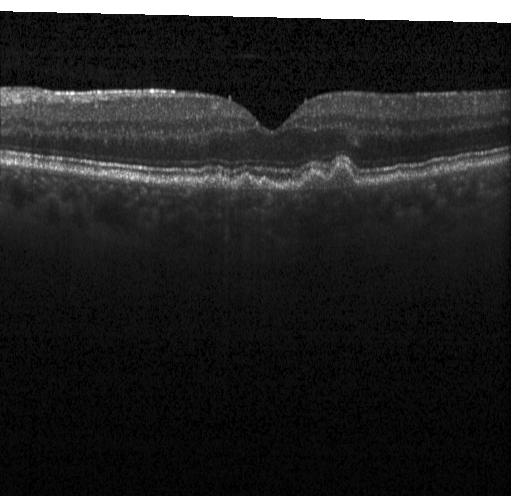
Retinal OCT B-scan
Impression: multiple drusen.